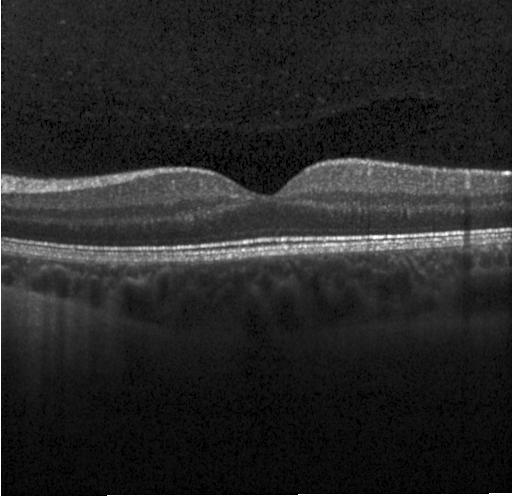
Heidelberg Spectralis OCT system. Retinal OCT B-scan. Macular scan
Finding: no choroidal neovascularization, no diabetic macular edema, and no drusen.